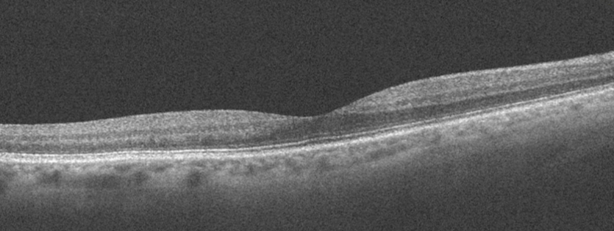
Optical coherence tomography B-scan, macular scan — Assessment: no evidence of AMD, DME, ERM, RAO, RVO, or VID.